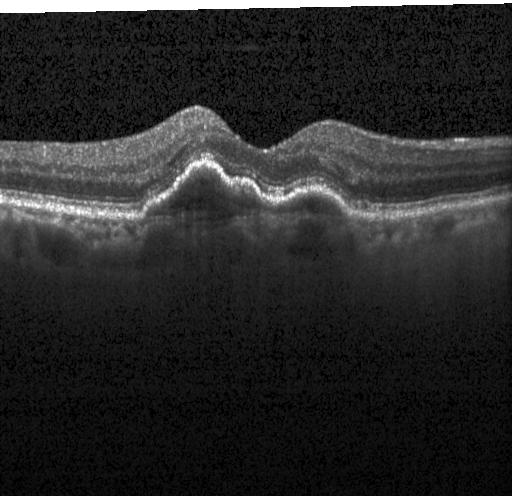

Horizontal scan through the fovea. Acquired on a Heidelberg Spectralis. Retinal OCT cross-section. Diagnosis: a choroidal neovascular membrane.